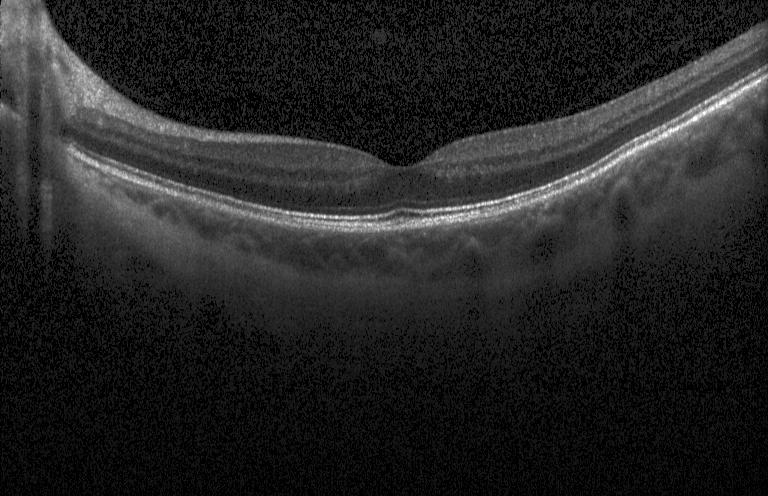

OCT B-scan; Heidelberg Spectralis OCT system; SD-OCT; through the macula — Macular OCT: no choroidal neovascularization, no diabetic macular edema, and no drusen.